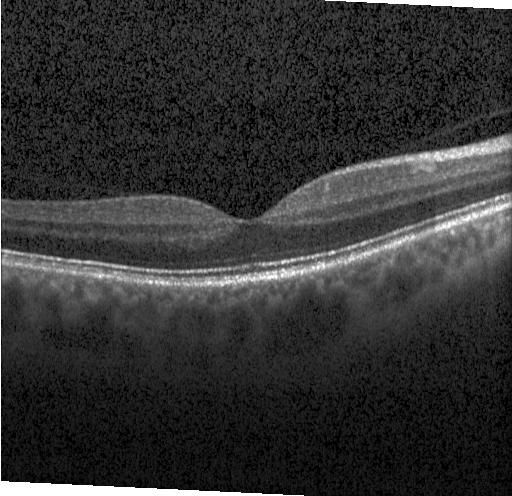 Horizontal scan through the fovea, OCT line scan, SD-OCT.
The scan shows no evidence of CNV, DME, or drusen.